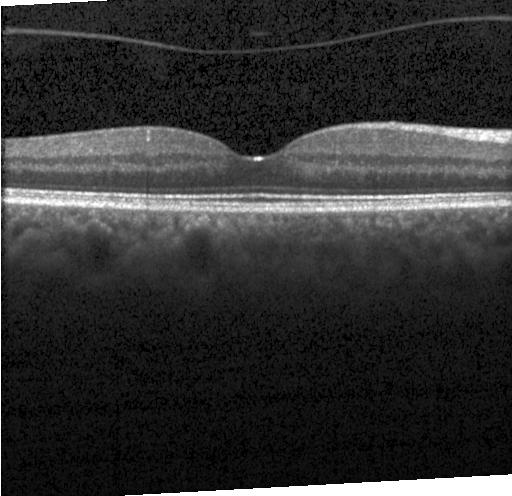 Macular scan; Heidelberg Spectralis OCT system; SD-OCT; optical coherence tomography scan
This B-scan demonstrates neither CNV, DME, nor drusen.